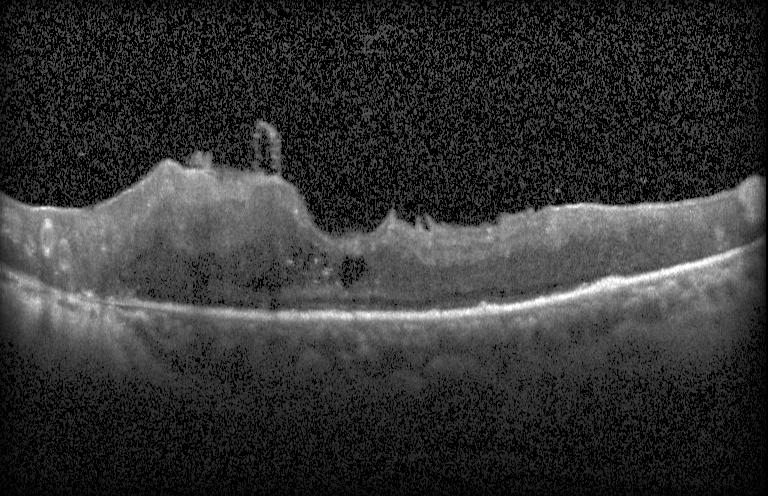
Centered on the fovea. Acquired on a Heidelberg Spectralis. OCT line scan — Impression: diabetic macular edema.